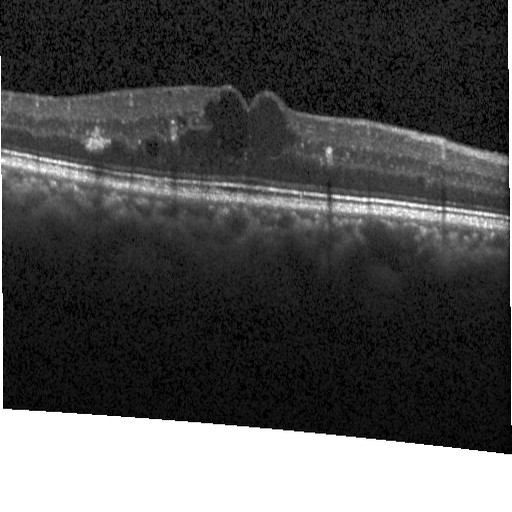 OCT B-scan — This B-scan demonstrates diabetic macular edema.